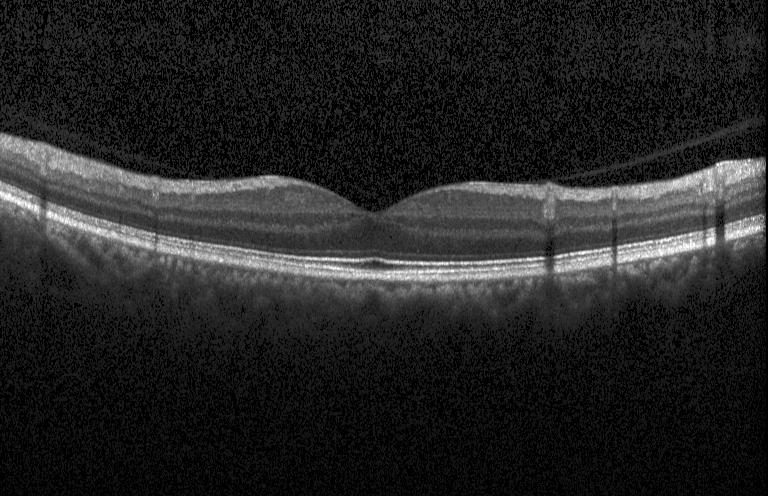 Spectral-domain OCT, retinal OCT cross-section — This B-scan demonstrates no evidence of choroidal neovascularization, diabetic macular edema, or drusen.